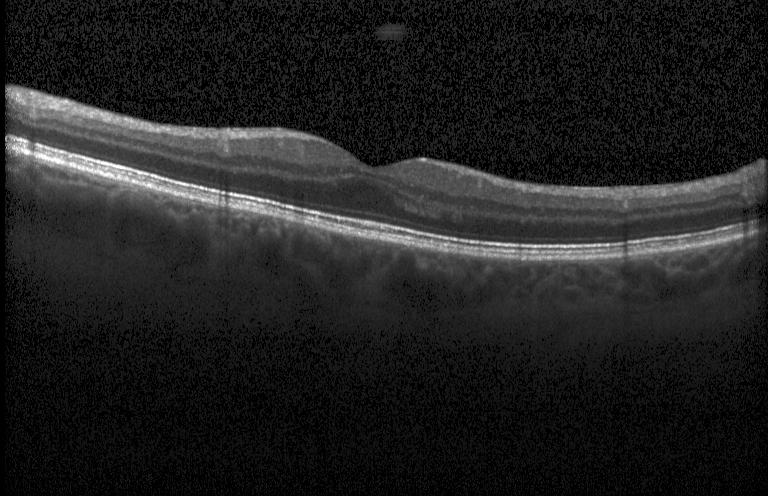 This B-scan demonstrates no choroidal neovascularization, no diabetic macular edema, and no drusen.